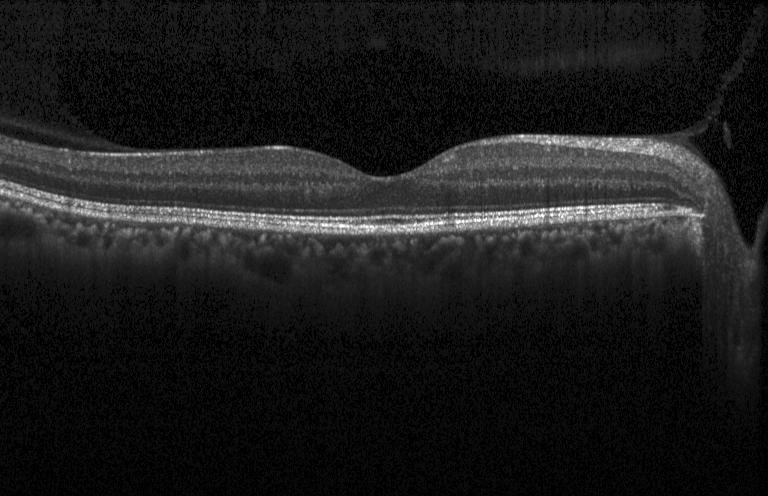 OCT B-scan. Acquired on a Heidelberg Spectralis.
Dx: neither choroidal neovascularization, diabetic macular edema, nor drusen.